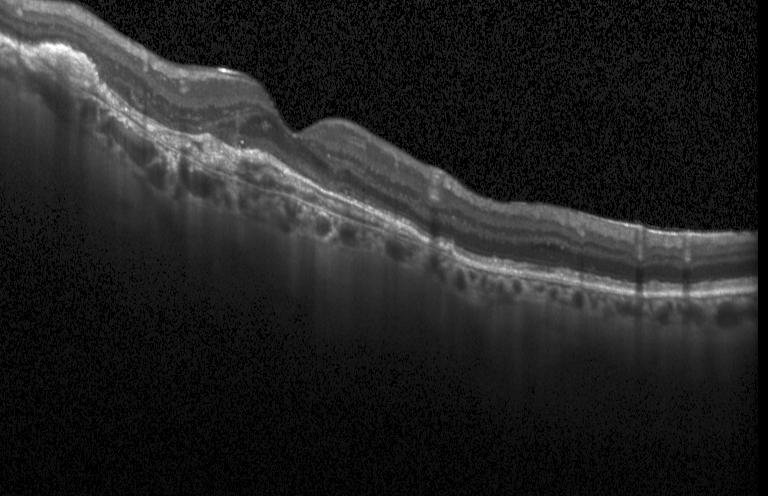 OCT line scan, spectral-domain optical coherence tomography.
Finding: choroidal neovascularization (CNV).